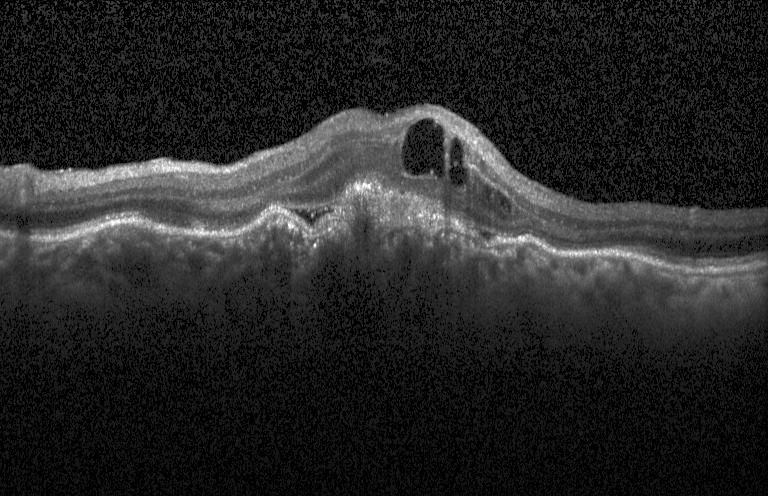 The scan shows choroidal neovascularization (CNV).